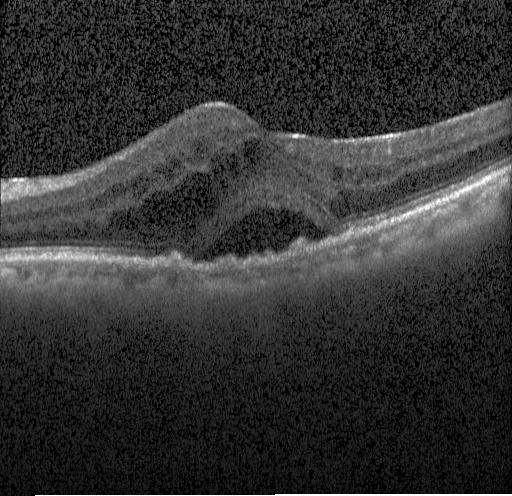

Optical coherence tomography scan.
Macular OCT: diabetic macular edema.